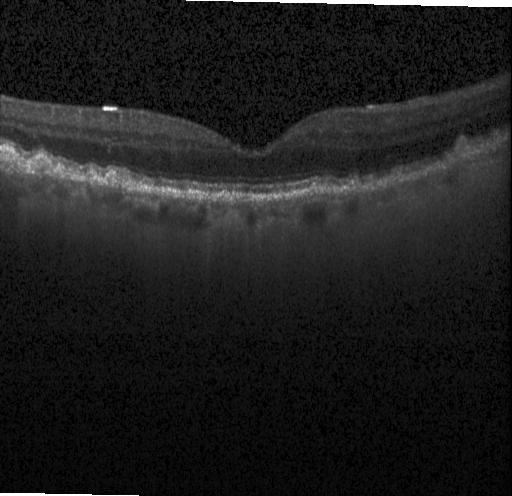

Retinal OCT B-scan; Heidelberg Spectralis OCT system; macular scan. Finding: drusen.